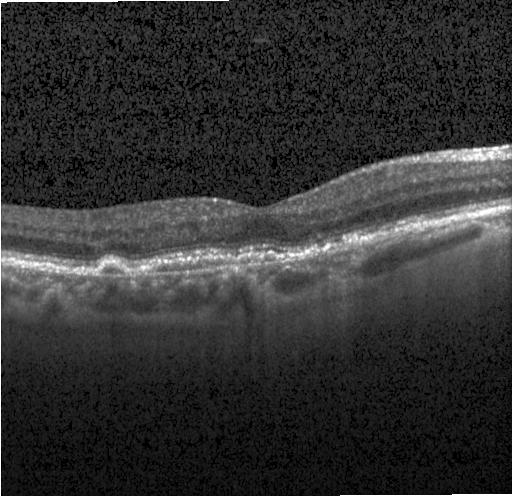
SD-OCT. Through the macula. OCT line scan. Finding: CNV.